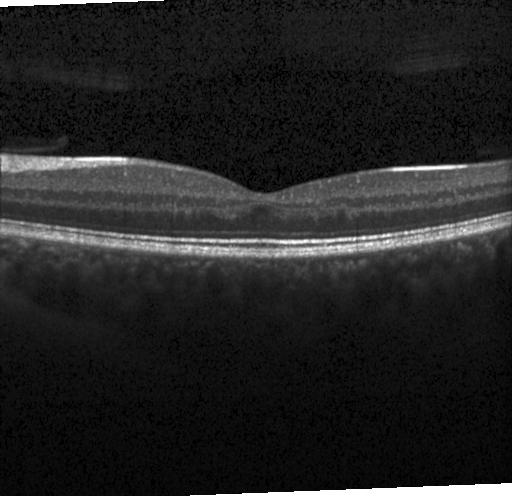
SD-OCT, instrument: Heidelberg Spectralis, OCT line scan, macular scan — Macular OCT: no CNV, no DME, and no drusen.